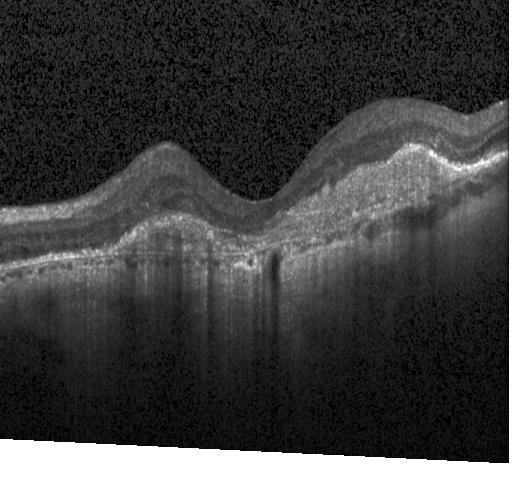 Retinal OCT cross-section; through the macula; spectral-domain OCT.
Dx: CNV.